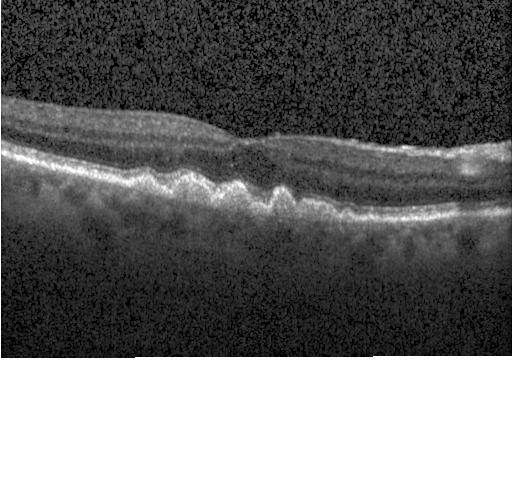

SD-OCT. Heidelberg Spectralis OCT system. Optical coherence tomography scan. Horizontal scan through the fovea.
Impression: drusen.